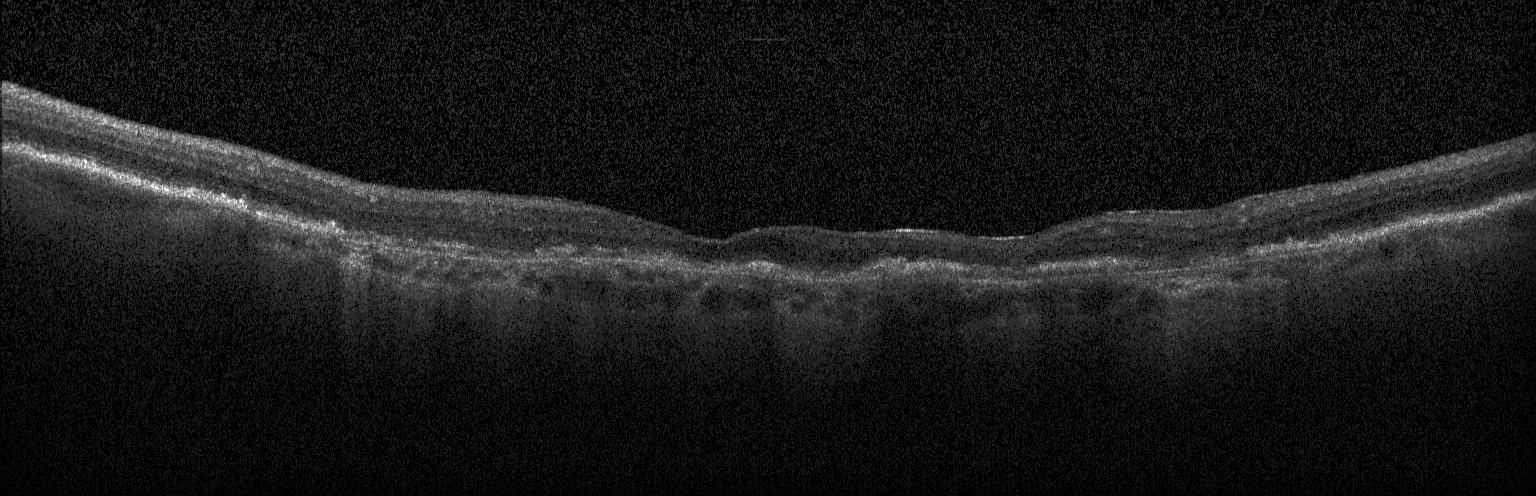

Retinal OCT B-scan. Macular scan. Acquired on a Heidelberg Spectralis. Impression: CNV.